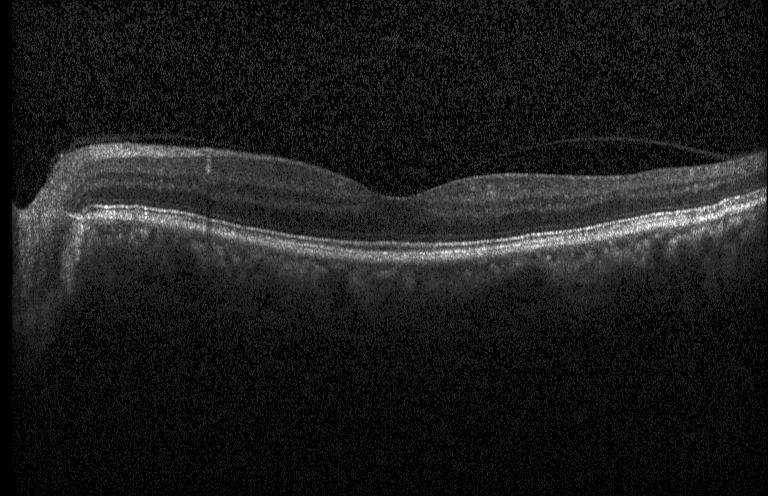 OCT B-scan · spectral-domain optical coherence tomography — Dx: no choroidal neovascularization, diabetic macular edema, or drusen.